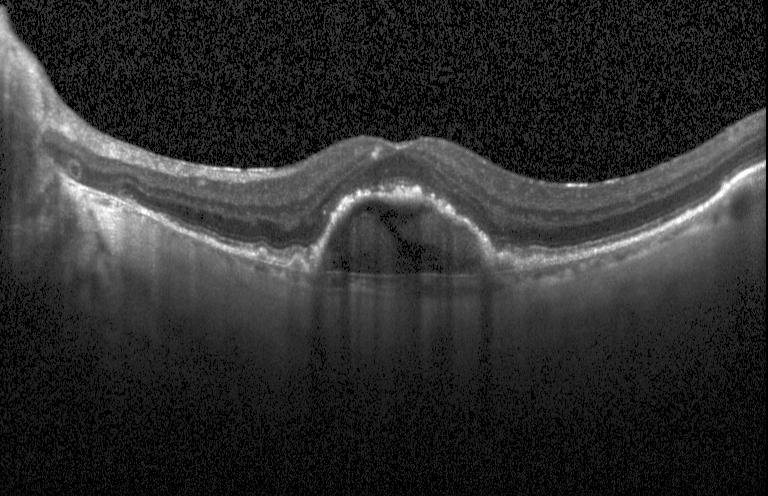
Diagnosis: a choroidal neovascular membrane.